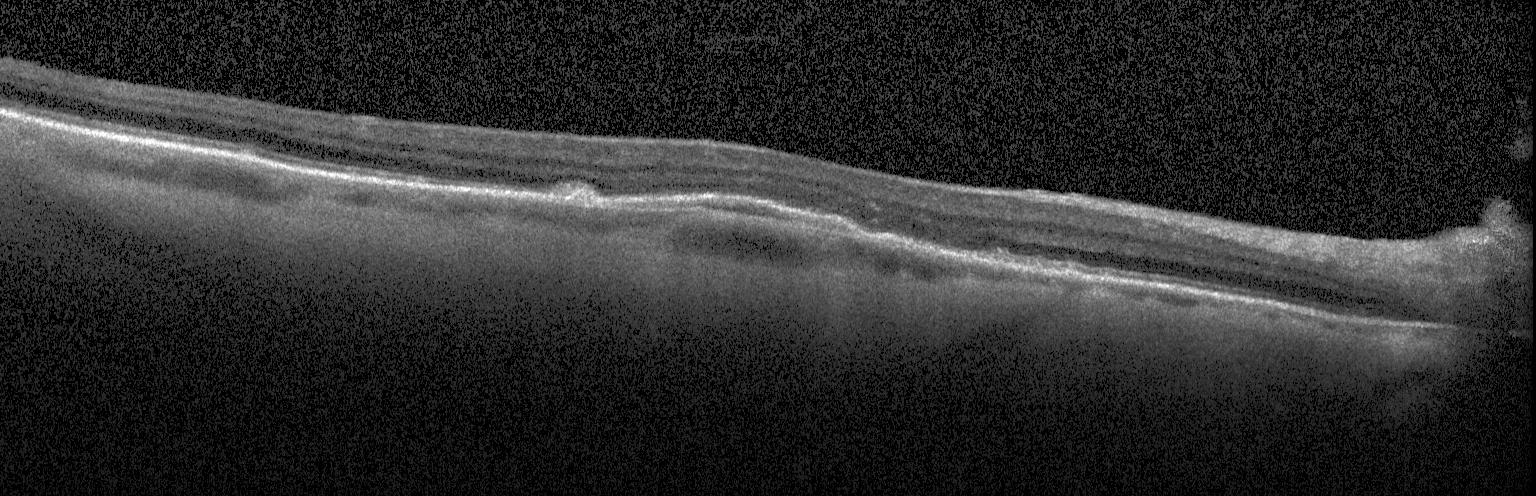 Retinal OCT cross-section. Dx: choroidal neovascularization (CNV).